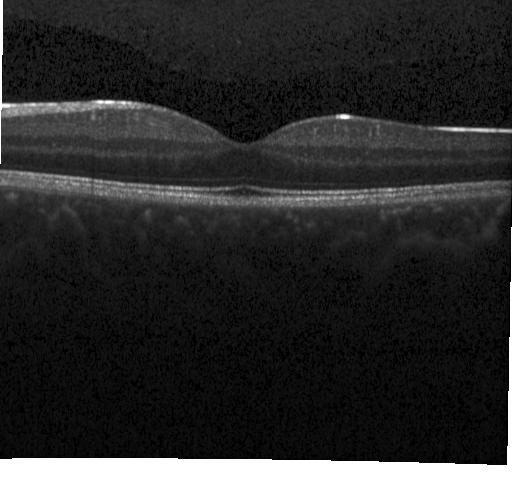 Optical coherence tomography B-scan · acquired on a Heidelberg Spectralis · fovea-centered · spectral-domain OCT — This B-scan demonstrates no choroidal neovascularization, diabetic macular edema, or drusen.